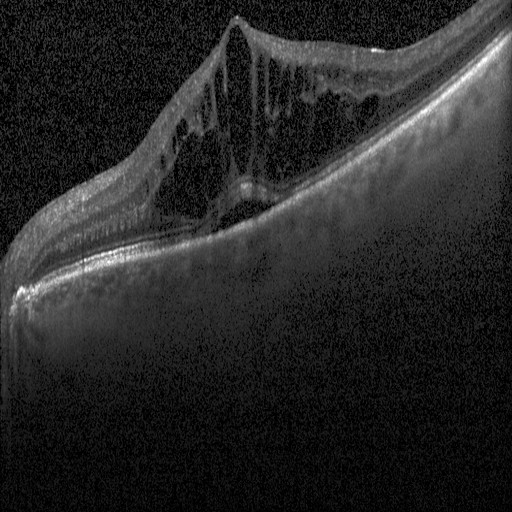
Spectral-domain OCT · optical coherence tomography B-scan. This B-scan demonstrates diabetic macular edema (DME).